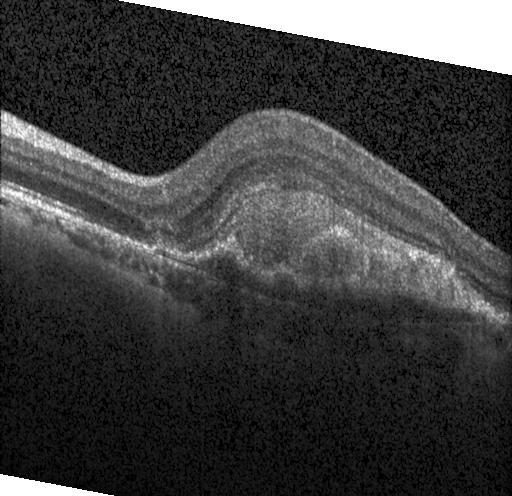 OCT line scan. This B-scan demonstrates a choroidal neovascular membrane.